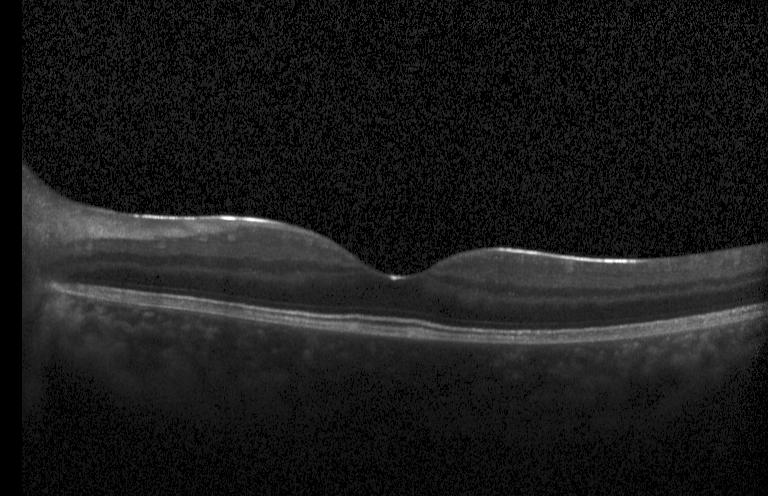

Retinal OCT cross-section showing neither CNV, DME, nor drusen.